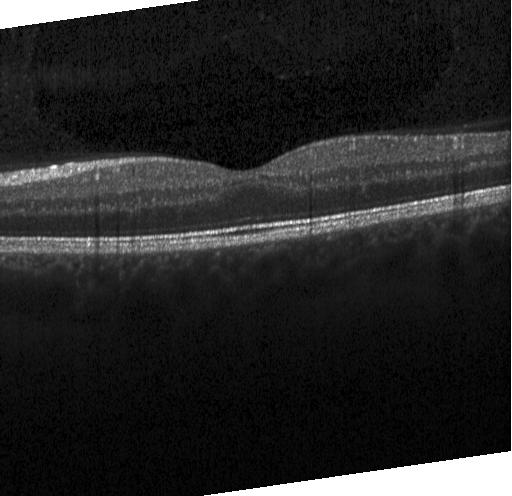 Optical coherence tomography scan. Fovea-centered. SD-OCT
Finding: no choroidal neovascularization, no diabetic macular edema, and no drusen.